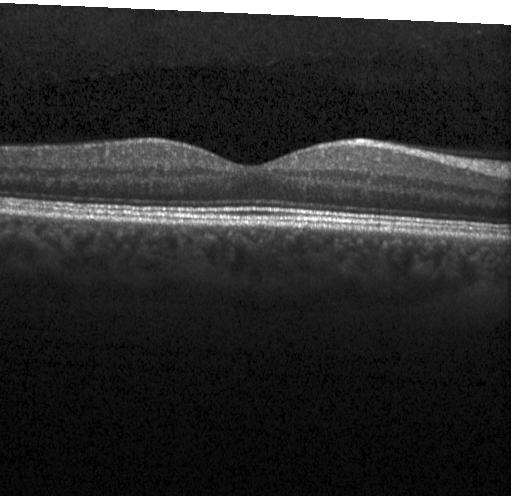

This B-scan demonstrates no evidence of choroidal neovascularization, diabetic macular edema, or drusen.